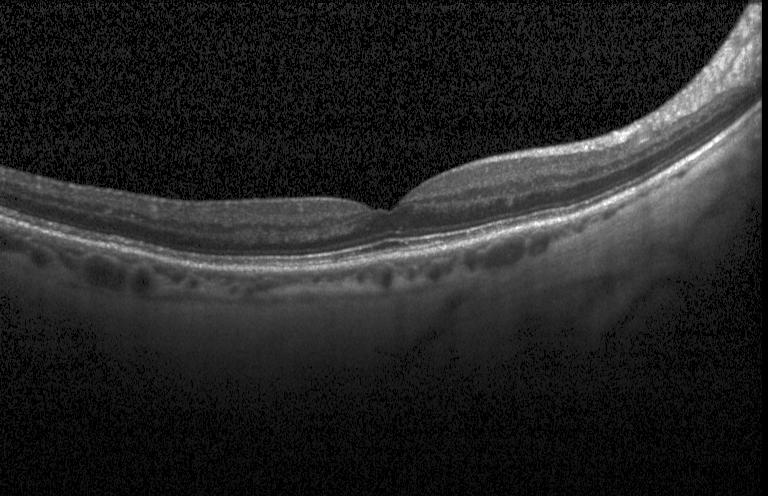
Optical coherence tomography scan — Impression: no evidence of CNV, DME, or drusen.